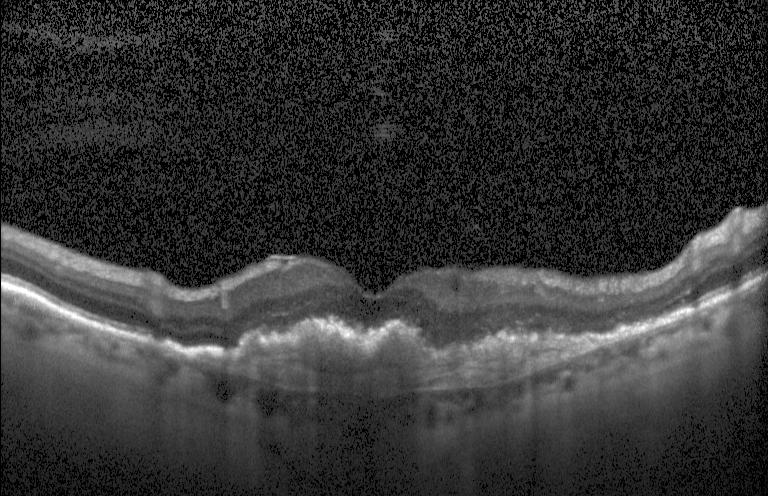
Finding: a choroidal neovascular membrane.